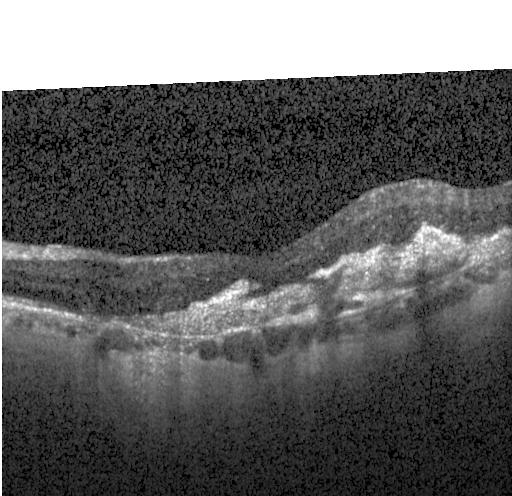

Retinal OCT cross-section. Assessment: CNV.